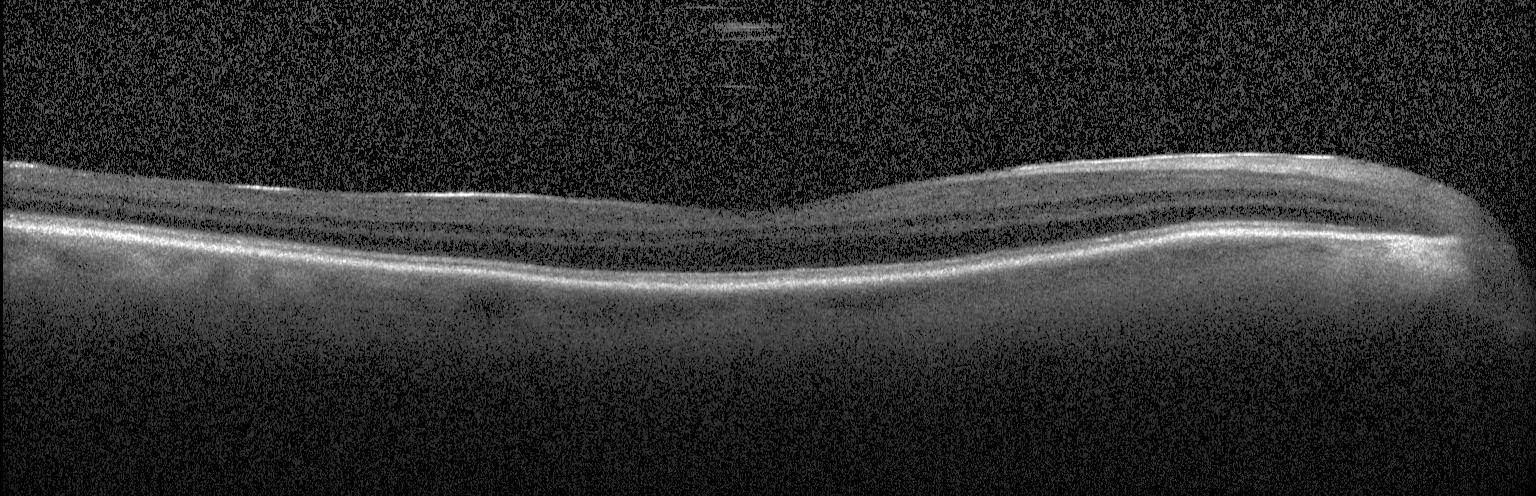
Optical coherence tomography B-scan. Spectral-domain optical coherence tomography. Fovea-centered.
This B-scan demonstrates no CNV, DME, or drusen.